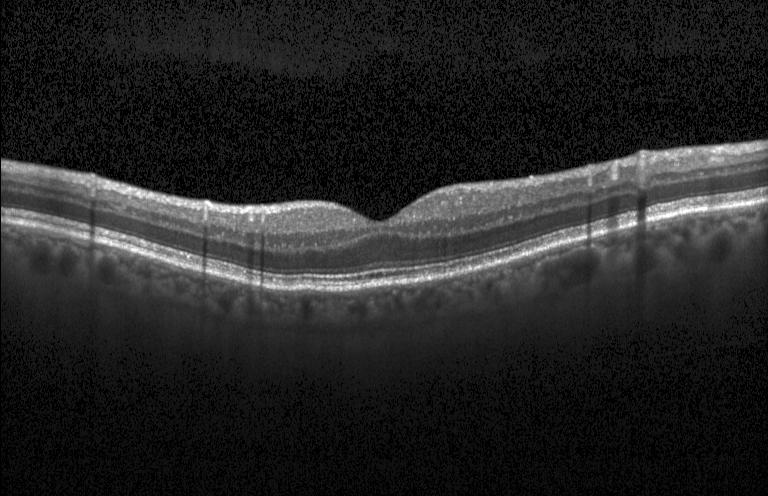

Macular OCT: no choroidal neovascularization, no diabetic macular edema, and no drusen.